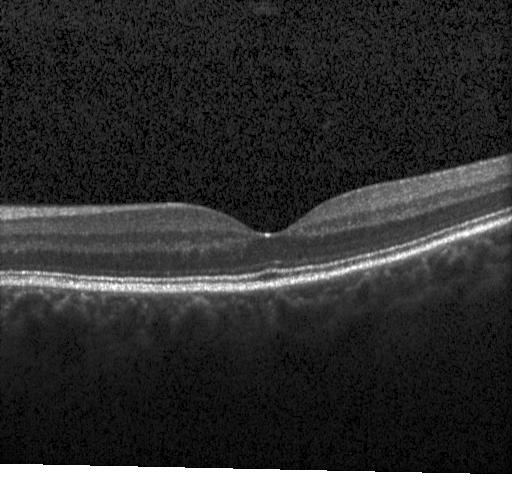

OCT finding: no evidence of choroidal neovascularization, diabetic macular edema, or drusen.